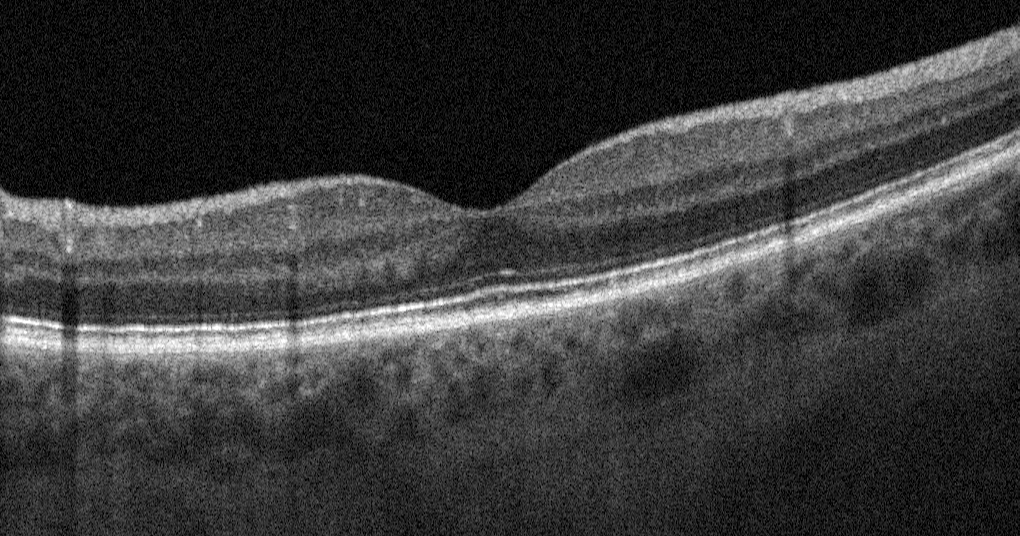
Optovue Avanti RTVue XR · retinal OCT B-scan · macular scan
Assessment: no evidence of AMD, DME, ERM, RAO, RVO, or VID.